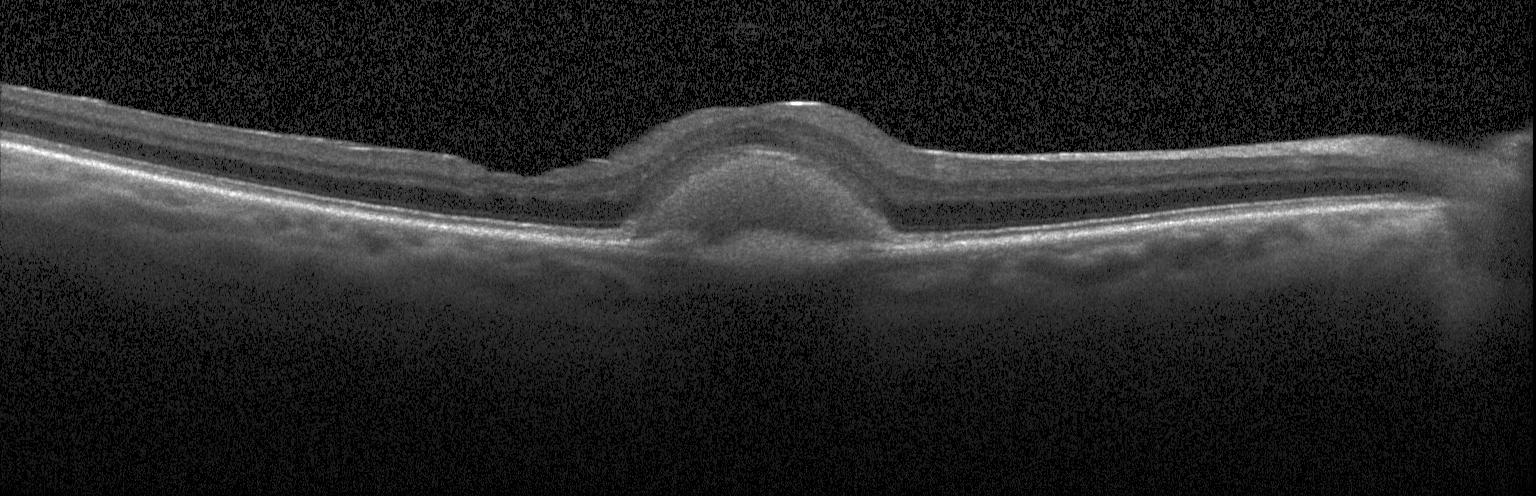

Impression: a choroidal neovascular membrane.